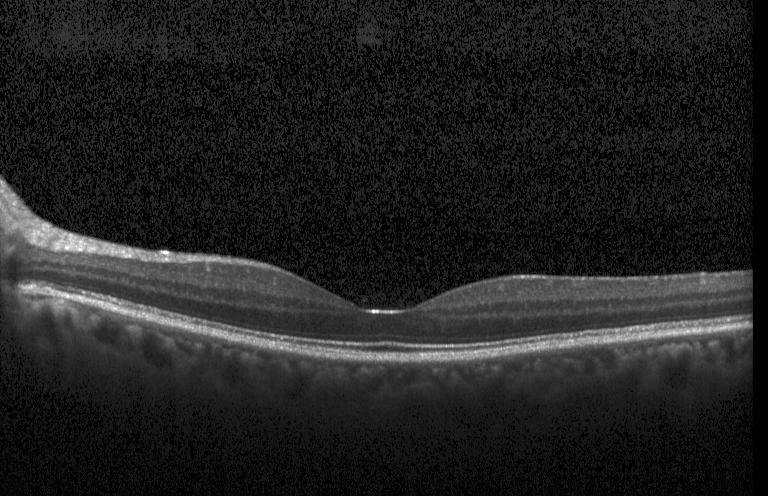

Retinal OCT cross-section · centered on the fovea — Diagnosis: no CNV, DME, or drusen.